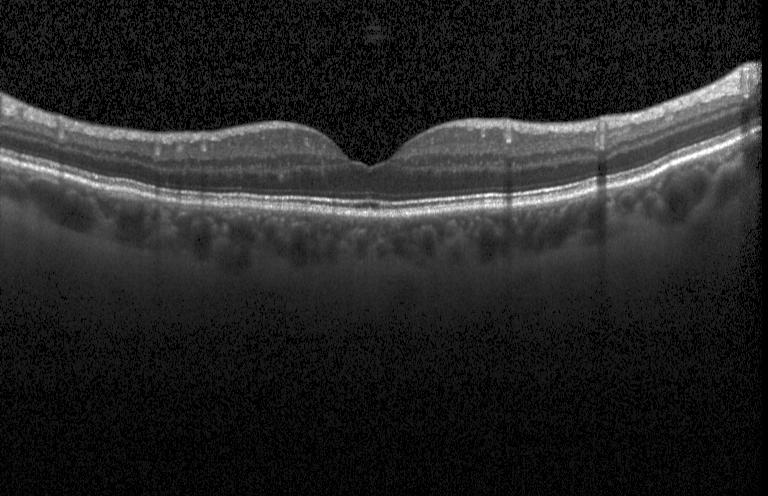

Macular OCT demonstrating neither choroidal neovascularization, diabetic macular edema, nor drusen.